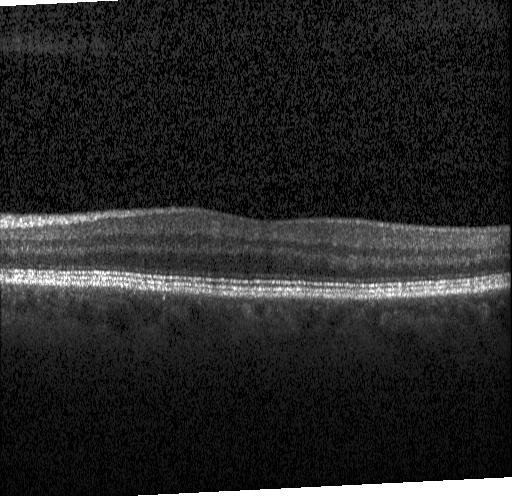
Acquired on a Heidelberg Spectralis. OCT B-scan. Impression: no choroidal neovascularization, no diabetic macular edema, and no drusen.